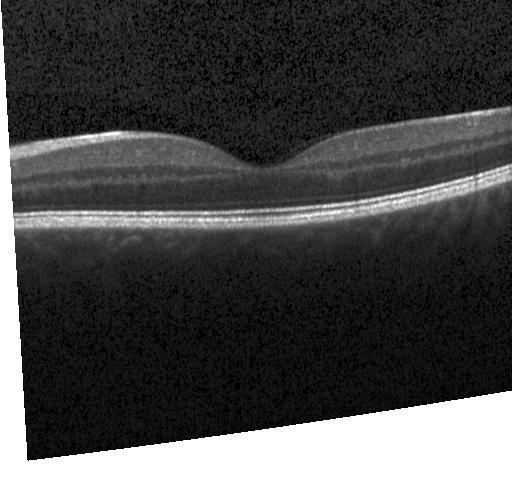 Macular OCT: no evidence of CNV, DME, or drusen.